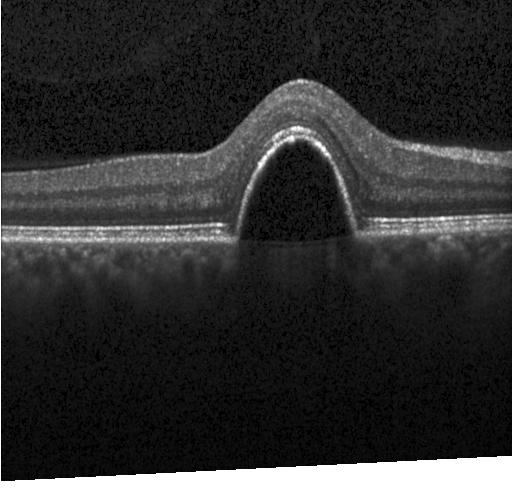 OCT finding: a choroidal neovascular membrane.